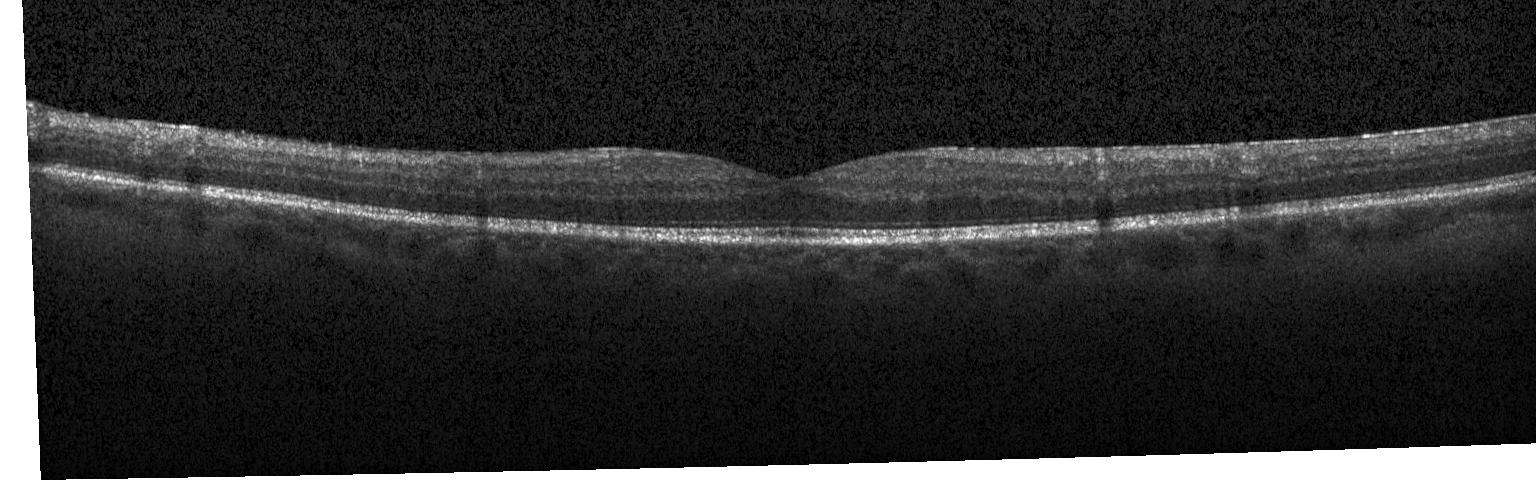

Impression: neither choroidal neovascularization, diabetic macular edema, nor drusen.